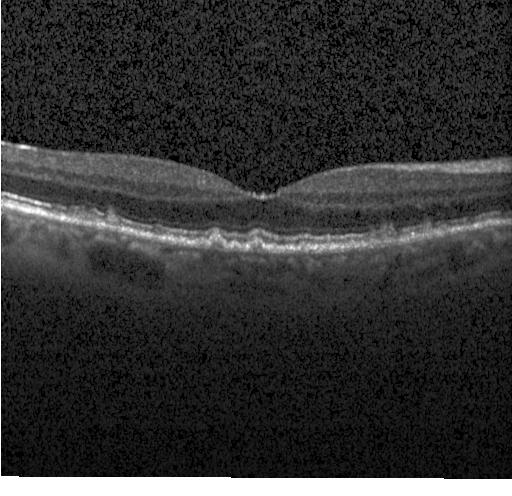 Through the macula; optical coherence tomography scan. This B-scan demonstrates multiple drusen.